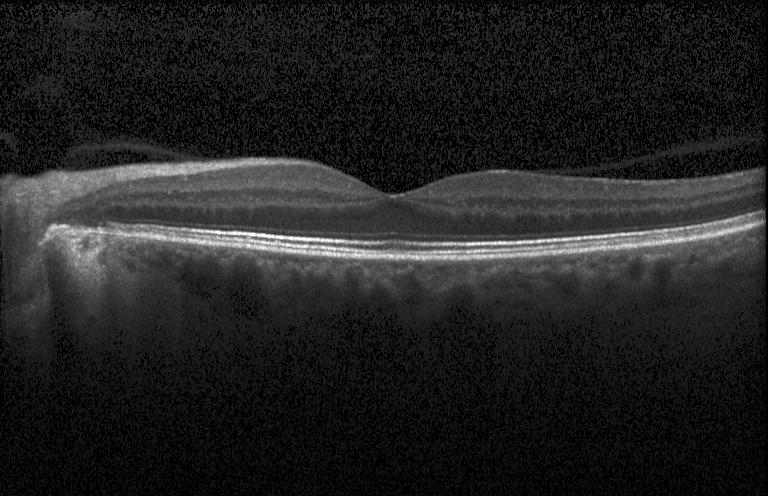

OCT finding: no CNV, DME, or drusen.